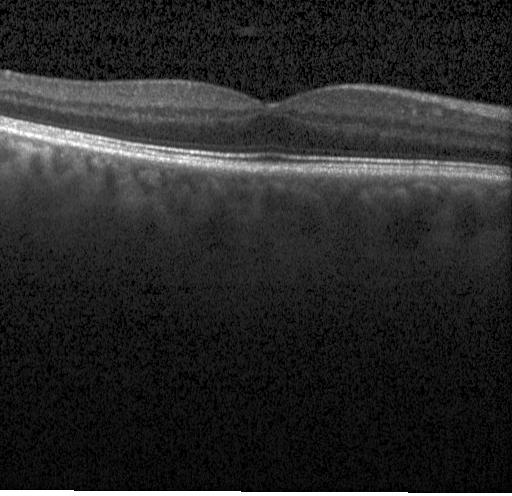
Centered on the fovea. Optical coherence tomography scan. Acquired on a Heidelberg Spectralis. Spectral-domain optical coherence tomography — Assessment: no CNV, DME, or drusen.